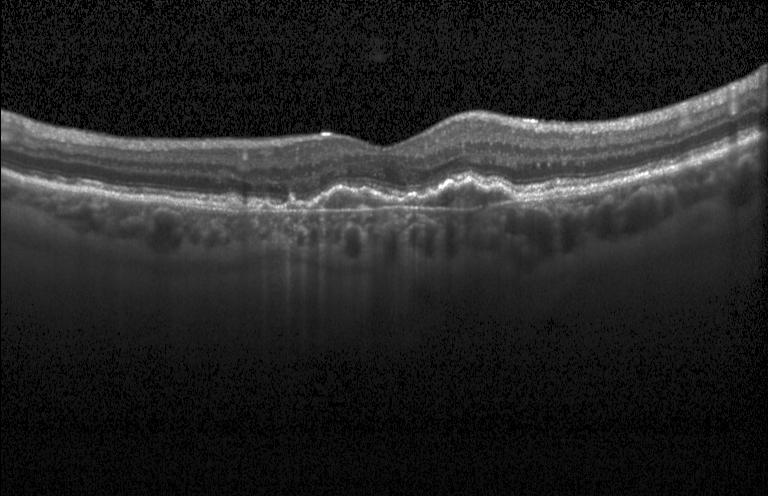

Acquired on a Heidelberg Spectralis, spectral-domain optical coherence tomography, retinal OCT cross-section
Diagnosis: choroidal neovascularization (CNV).